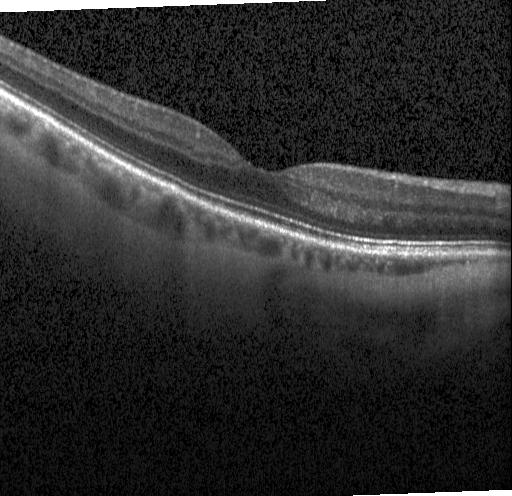 Diagnosis: neither choroidal neovascularization, diabetic macular edema, nor drusen.